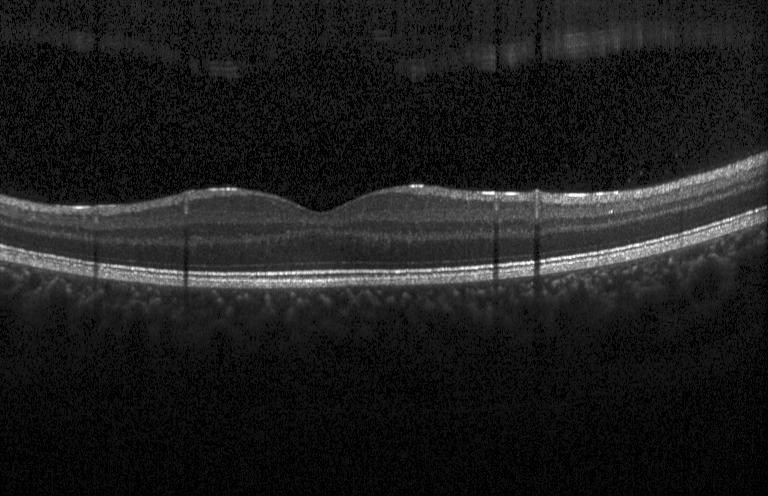

SD-OCT, retinal OCT cross-section, through the macula, acquired on a Heidelberg Spectralis — This B-scan demonstrates no evidence of choroidal neovascularization, diabetic macular edema, or drusen.